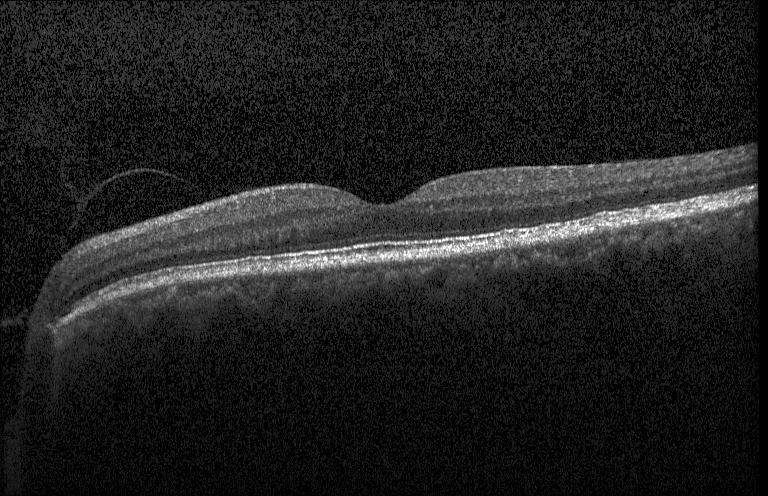
OCT scan showing neither choroidal neovascularization, diabetic macular edema, nor drusen.